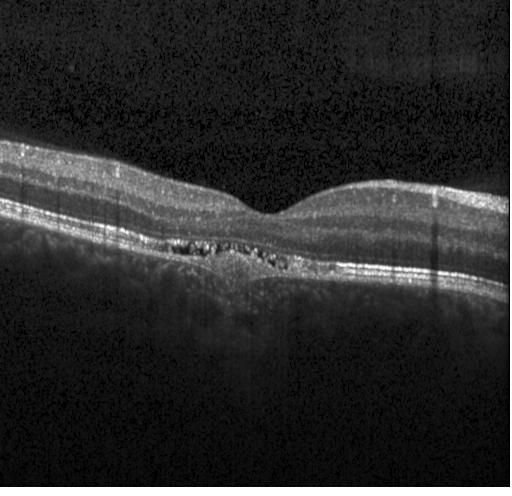
OCT line scan — Macular OCT: choroidal neovascularization.